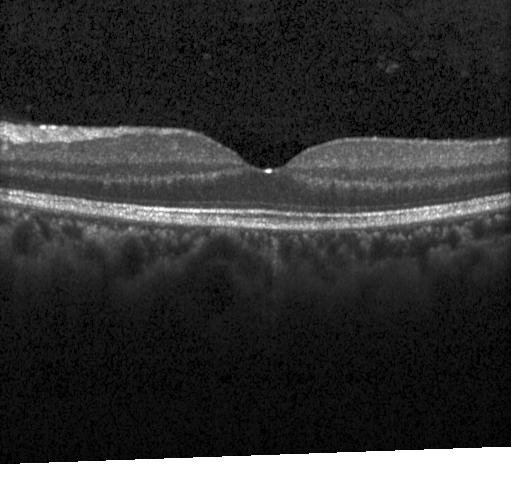 Retinal OCT cross-section
Impression: no CNV, no DME, and no drusen.